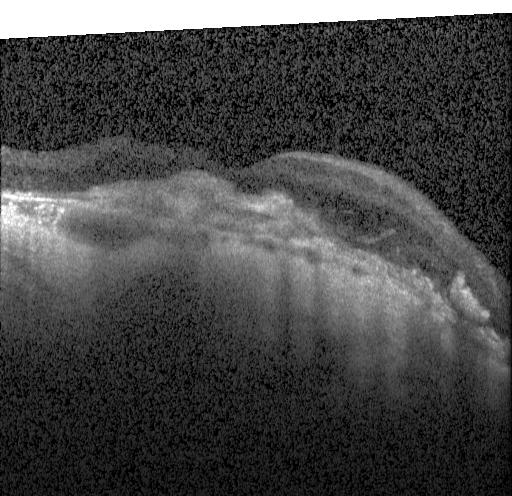

SD-OCT, OCT line scan.
Impression: CNV.